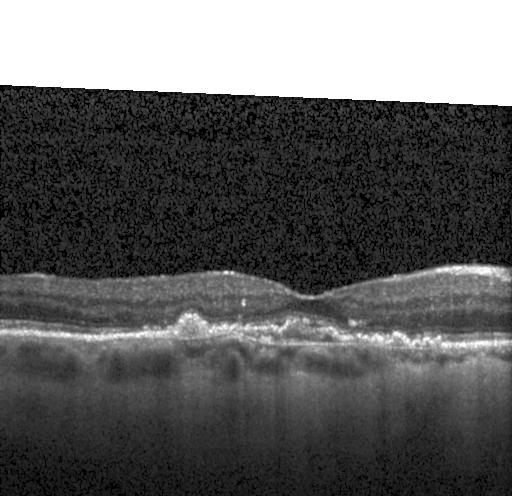

Acquired on a Heidelberg Spectralis, spectral-domain OCT, OCT line scan.
Assessment: a choroidal neovascular membrane.